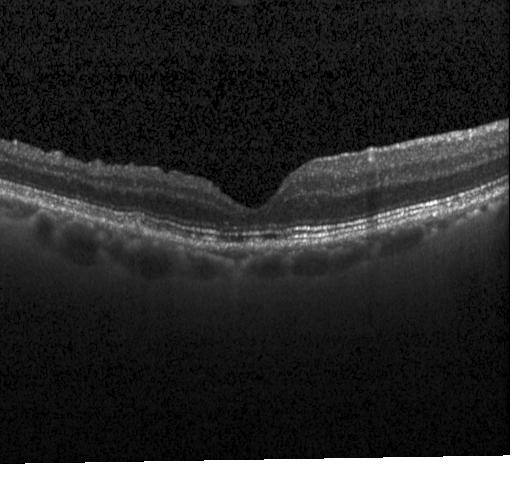 SD-OCT; retinal OCT cross-section; instrument: Heidelberg Spectralis
Diagnosis: no choroidal neovascularization, diabetic macular edema, or drusen.